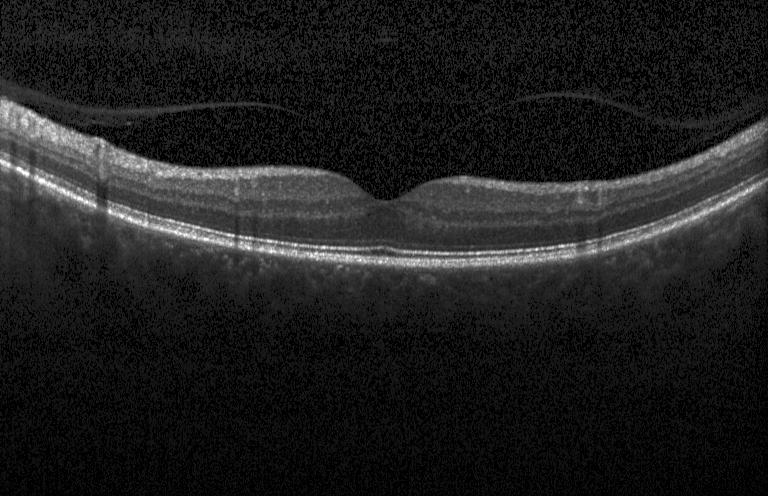
Retinal OCT B-scan. Neither choroidal neovascularization, diabetic macular edema, nor drusen.